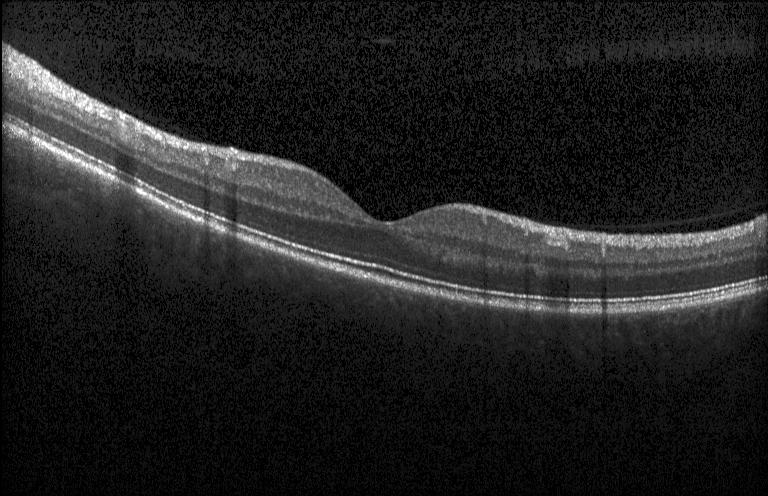

Retinal OCT cross-section, SD-OCT, horizontal scan through the fovea, Heidelberg Spectralis — Impression: neither choroidal neovascularization, diabetic macular edema, nor drusen.